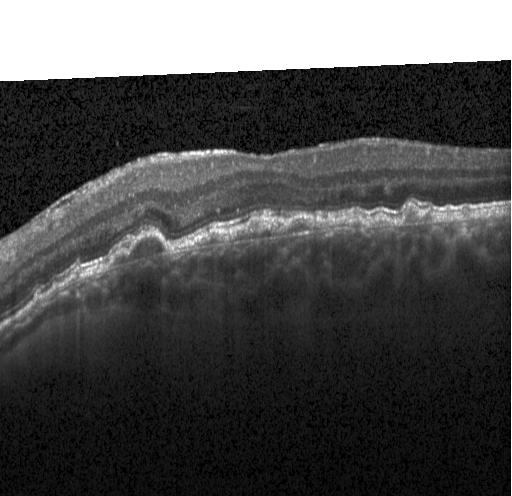

Finding: a choroidal neovascular membrane.